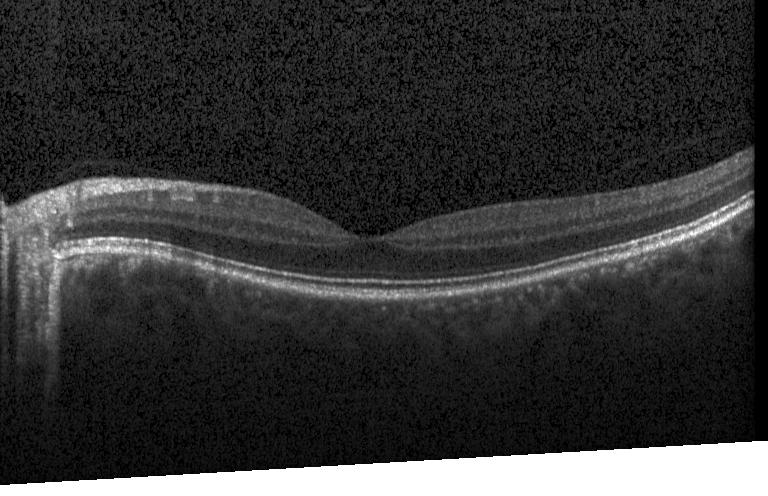 Retinal OCT cross-section, horizontal scan through the fovea. Dx: neither CNV, DME, nor drusen.